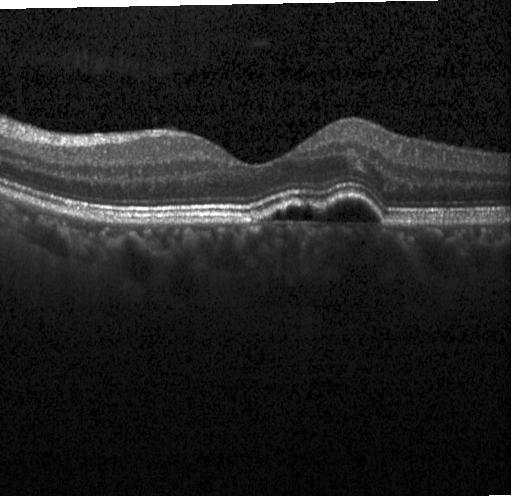 Macular OCT demonstrating a choroidal neovascular membrane.